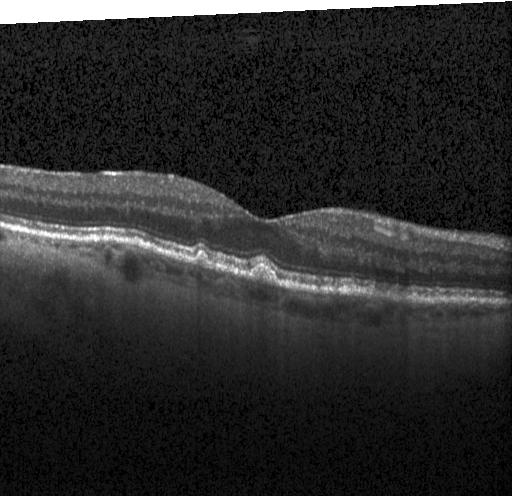

Finding: drusen.